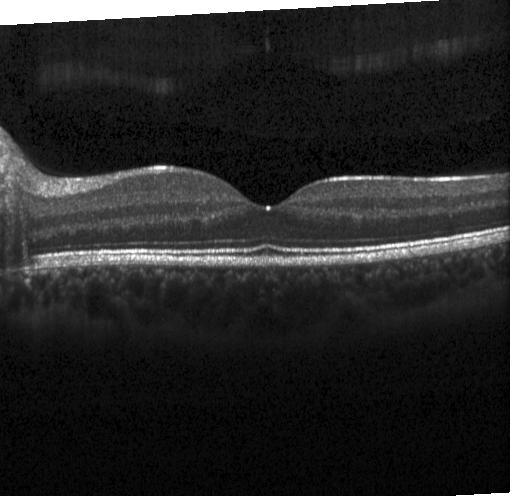

Heidelberg Spectralis, macular scan, OCT B-scan, spectral-domain optical coherence tomography — Finding: no CNV, no DME, and no drusen.